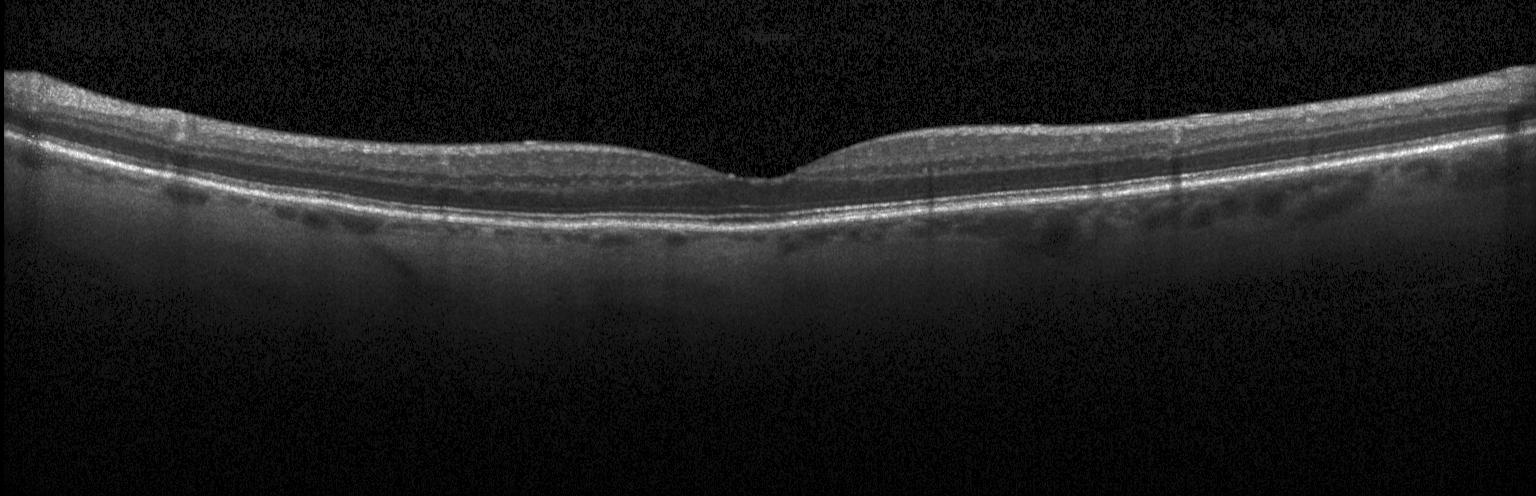 This B-scan demonstrates no evidence of choroidal neovascularization, diabetic macular edema, or drusen.